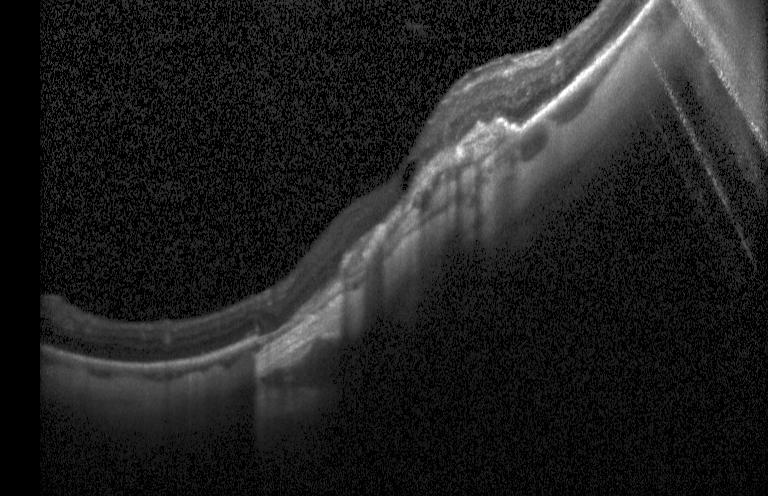
Dx: a choroidal neovascular membrane.